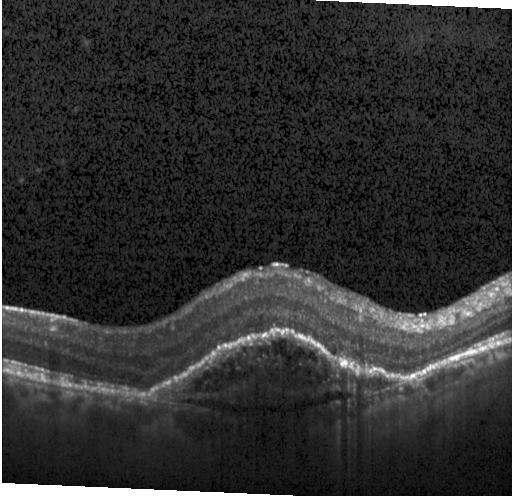
Optical coherence tomography B-scan. Finding: choroidal neovascularization (CNV).